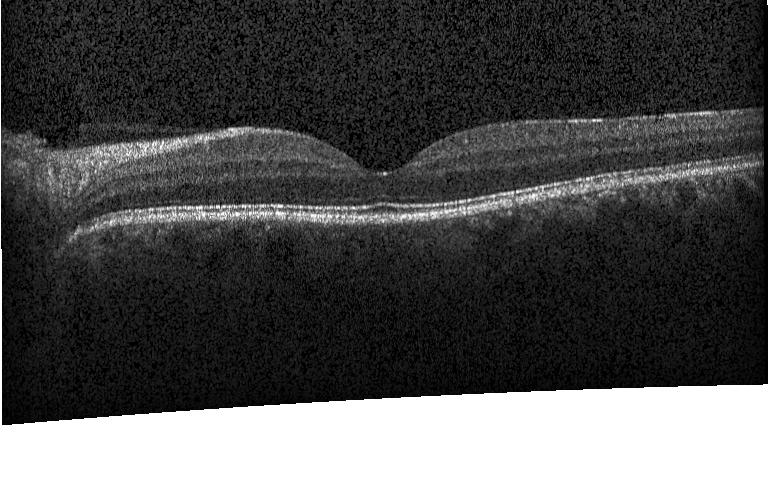 Impression: neither choroidal neovascularization, diabetic macular edema, nor drusen.